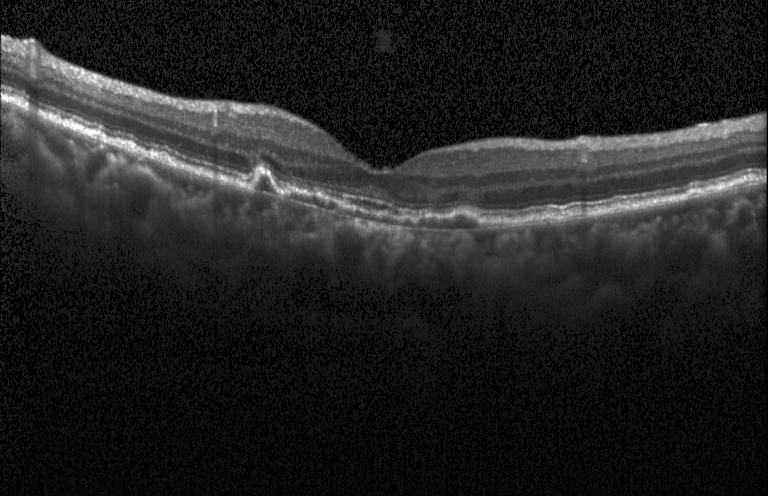
OCT line scan.
This B-scan demonstrates a choroidal neovascular membrane.